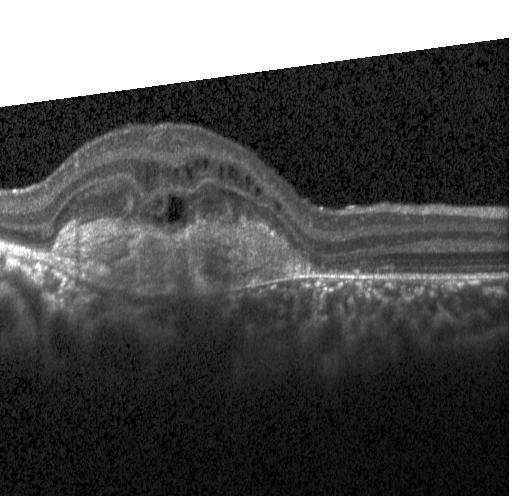
OCT line scan. Choroidal neovascularization (CNV).